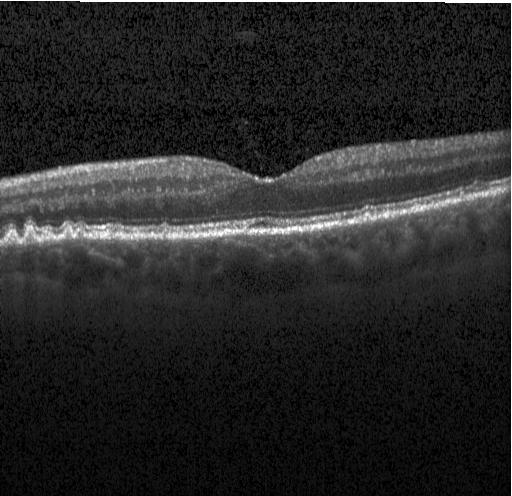

Spectral-domain OCT, optical coherence tomography B-scan
Finding: sub-RPE drusenoid deposits.